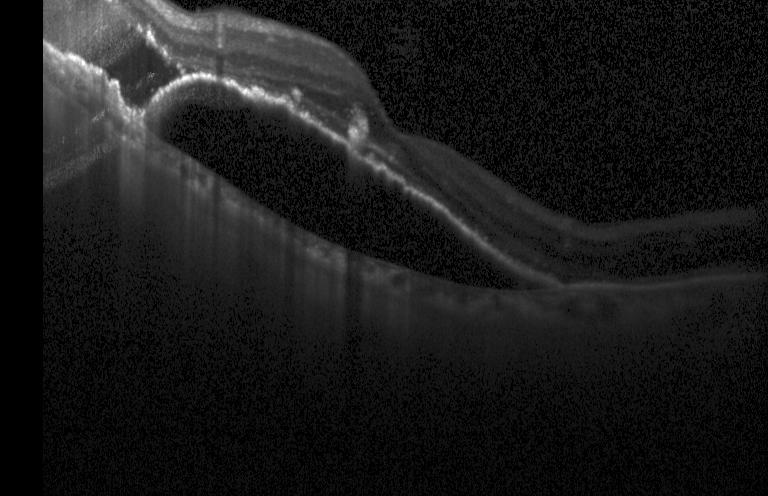
Optical coherence tomography B-scan; SD-OCT.
Dx: a choroidal neovascular membrane.